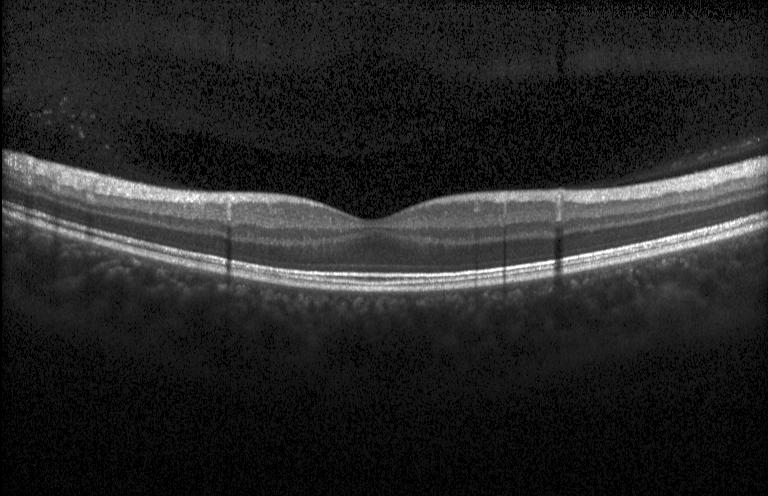 Through the macula; Heidelberg Spectralis OCT system; SD-OCT; retinal OCT cross-section. The scan shows neither choroidal neovascularization, diabetic macular edema, nor drusen.